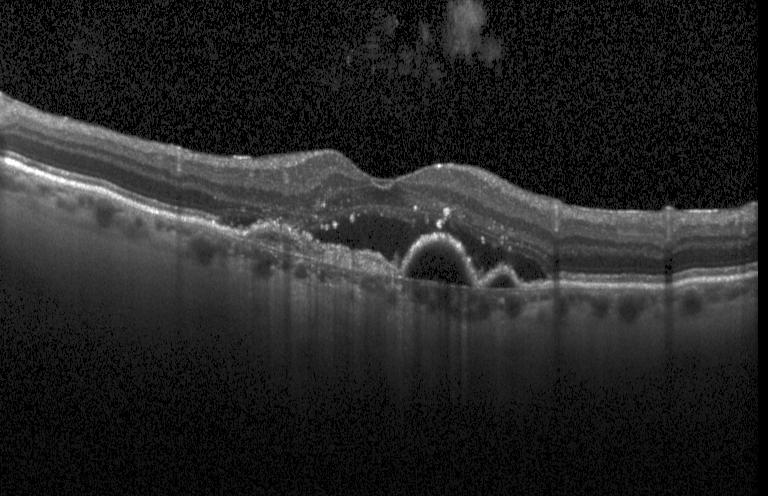
Spectral-domain OCT. Retinal OCT cross-section
Finding: CNV.